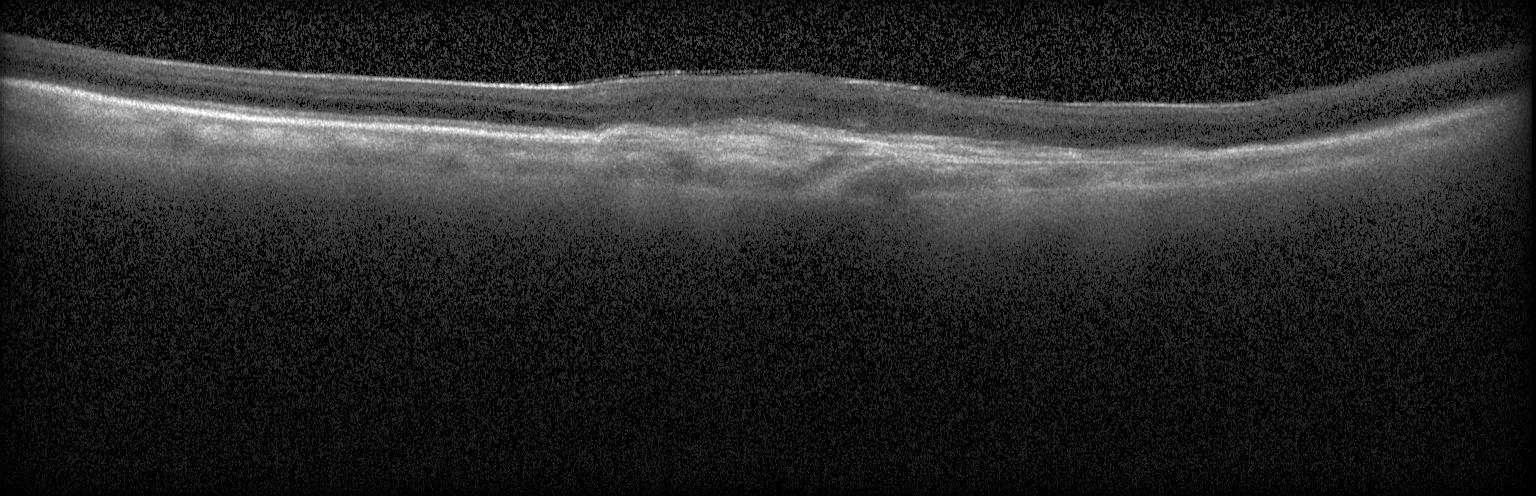
OCT B-scan showing CNV.